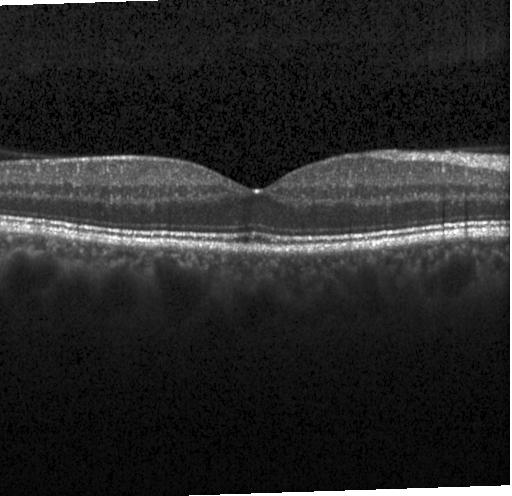
The scan shows no evidence of CNV, DME, or drusen.